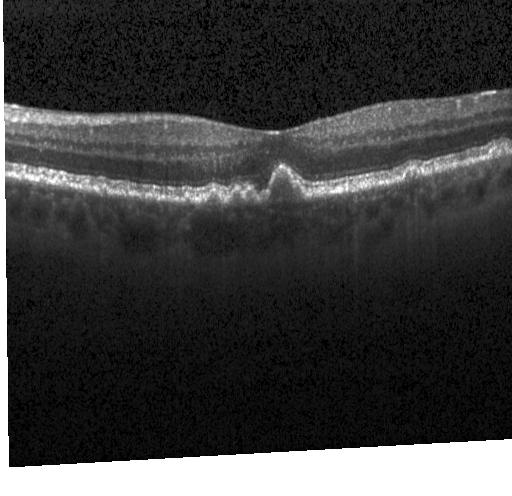
Spectral-domain OCT B-scan: drusen.